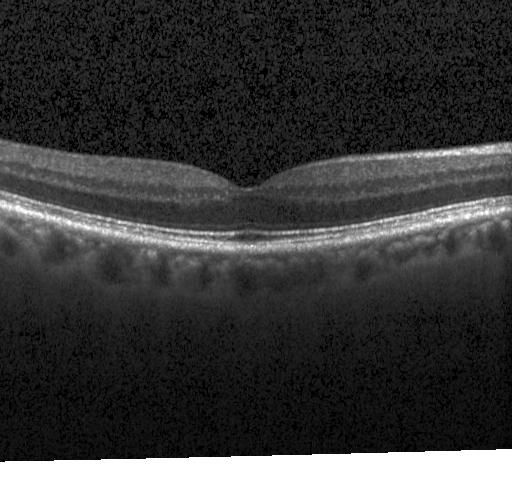
Fovea-centered; OCT line scan; SD-OCT
OCT finding: no CNV, DME, or drusen.